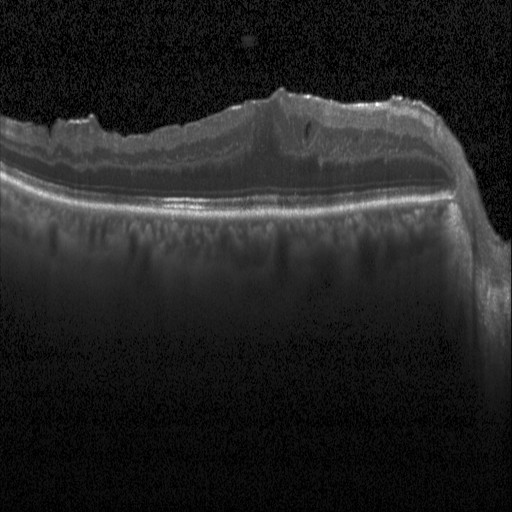

OCT B-scan showing DME.